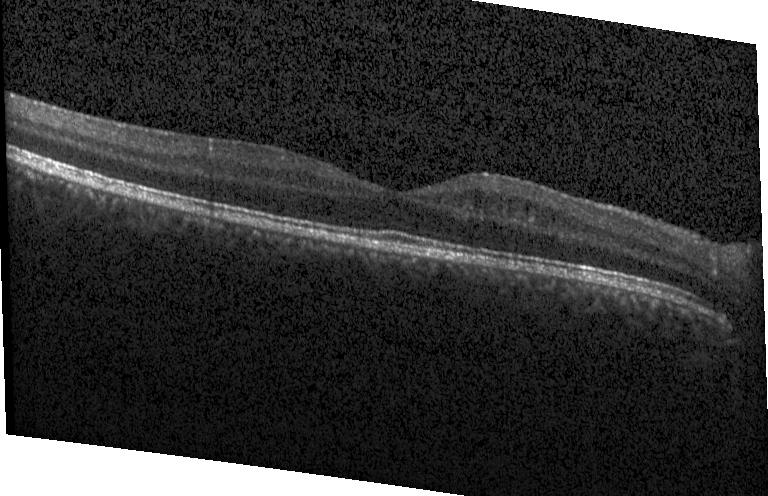 Heidelberg Spectralis OCT system · optical coherence tomography scan · macular scan — Diagnosis: DME.